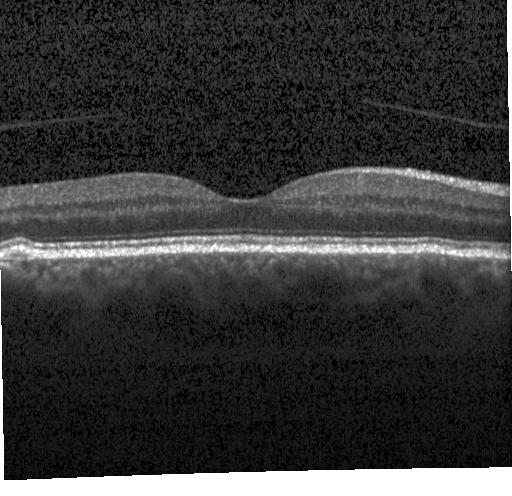 OCT finding: sub-RPE drusenoid deposits.